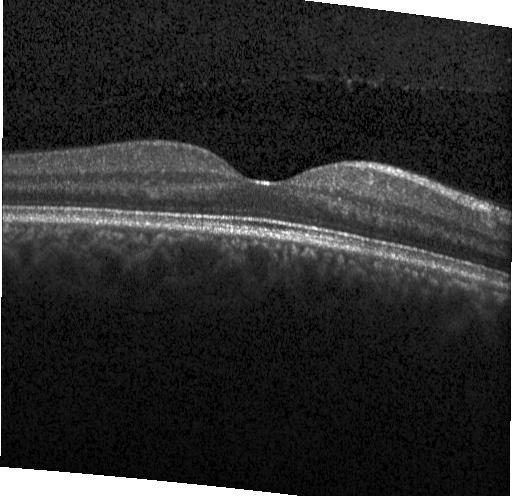
Retinal OCT B-scan.
No choroidal neovascularization, no diabetic macular edema, and no drusen.